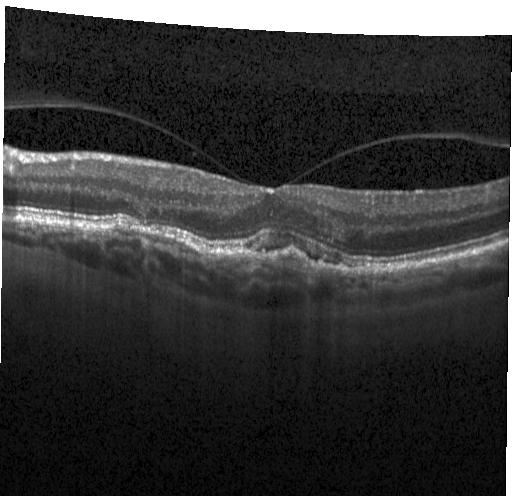 Retinal OCT cross-section
Finding: choroidal neovascularization.